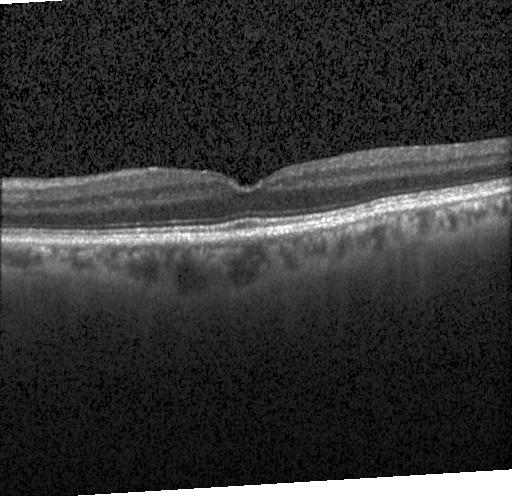

Dx: no choroidal neovascularization, diabetic macular edema, or drusen.